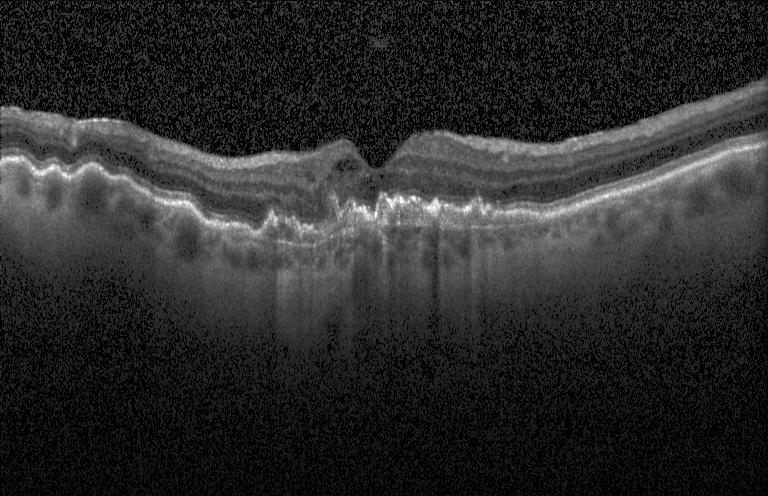

Impression: choroidal neovascularization (CNV).